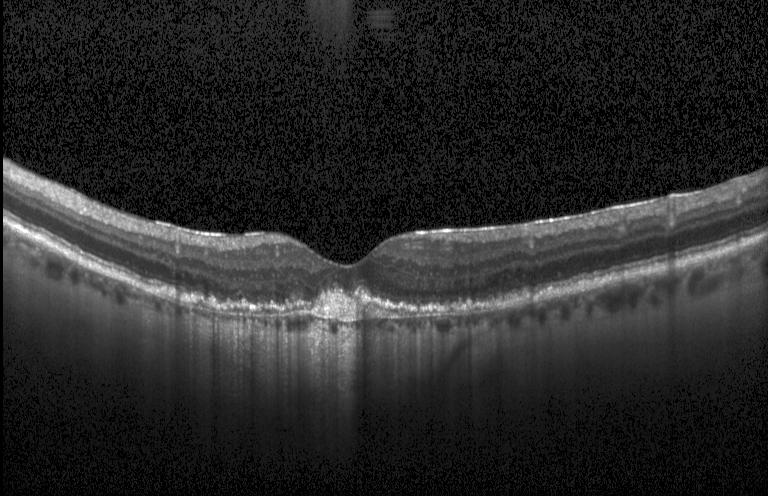
Macular scan, OCT B-scan
The scan shows choroidal neovascularization.